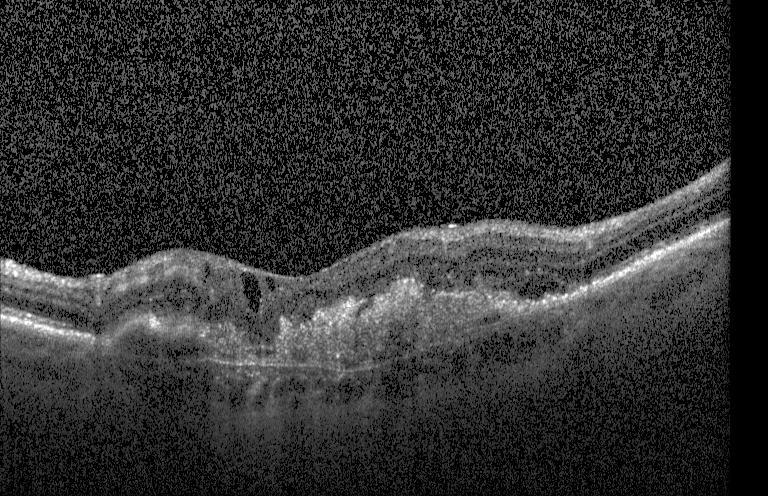

Centered on the fovea · instrument: Heidelberg Spectralis · spectral-domain optical coherence tomography · optical coherence tomography B-scan. Assessment: a choroidal neovascular membrane.